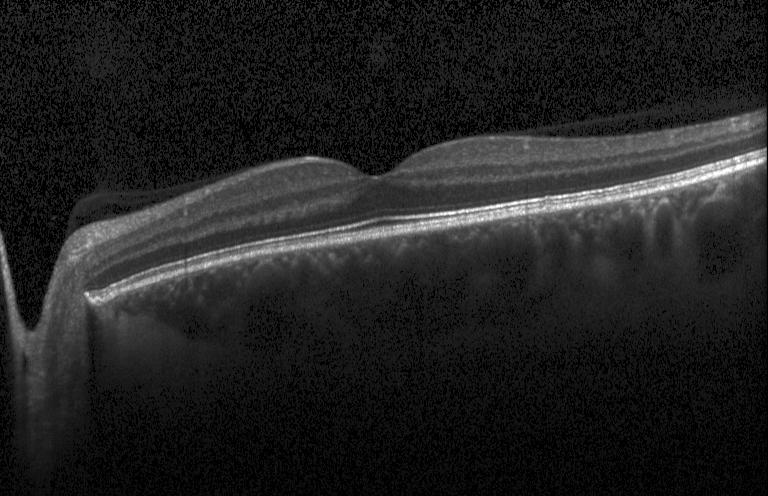
This B-scan demonstrates neither choroidal neovascularization, diabetic macular edema, nor drusen.